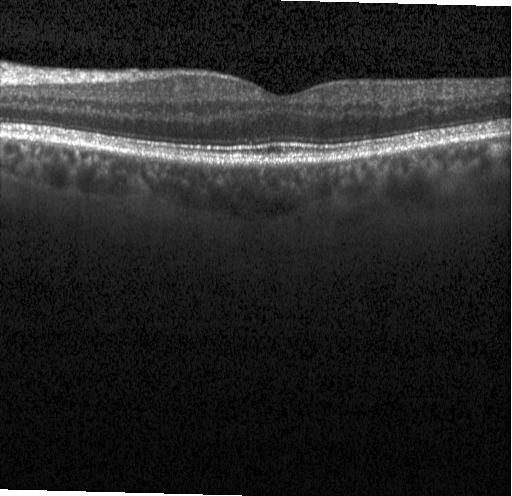
Spectral-domain OCT, through the macula, optical coherence tomography scan — This B-scan demonstrates no evidence of choroidal neovascularization, diabetic macular edema, or drusen.